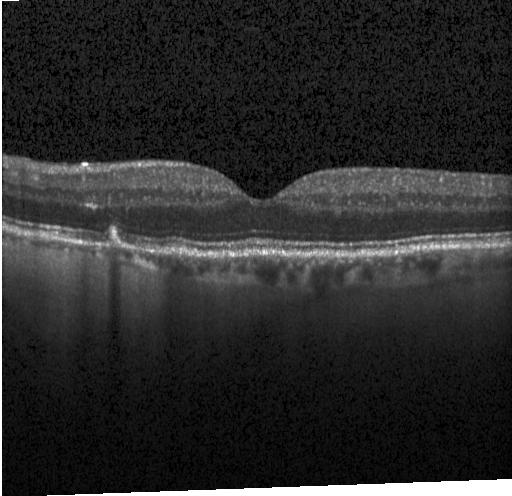

Macular scan; OCT line scan.
Finding: multiple drusen.